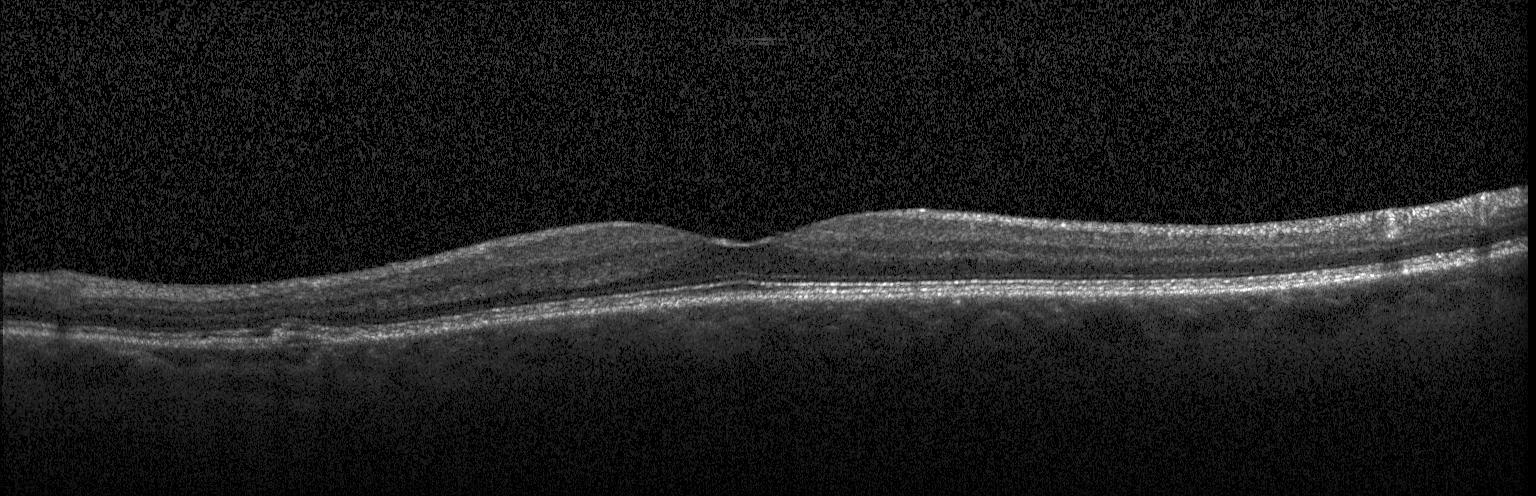 Optical coherence tomography scan
The scan shows multiple drusen.